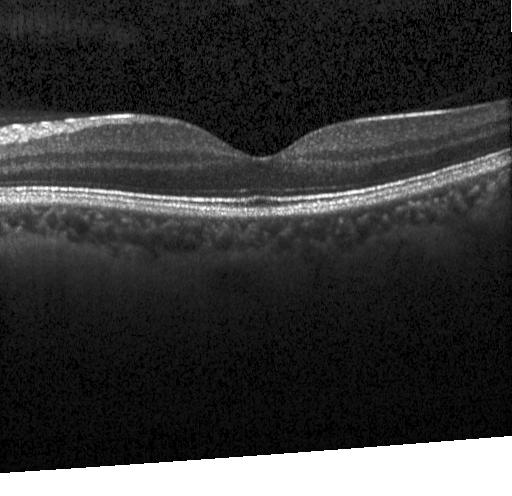 Instrument: Heidelberg Spectralis · spectral-domain OCT · retinal OCT B-scan · centered on the fovea.
Macular OCT: no choroidal neovascularization, no diabetic macular edema, and no drusen.